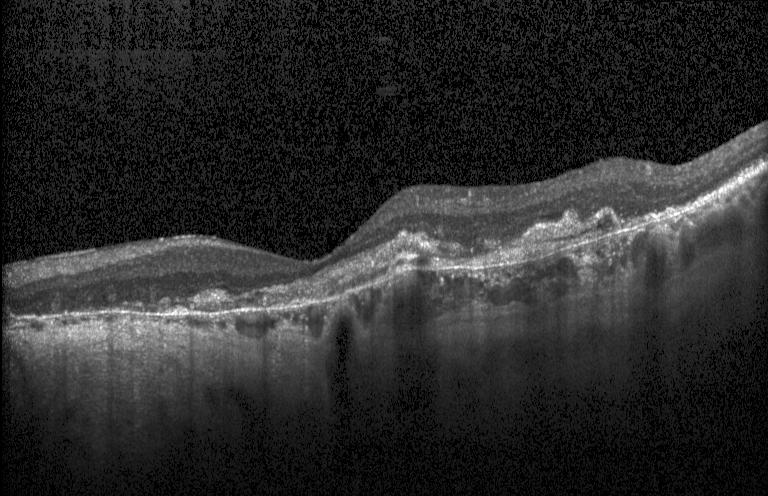 Horizontal scan through the fovea, OCT line scan, Heidelberg Spectralis, spectral-domain OCT.
The scan shows a choroidal neovascular membrane.